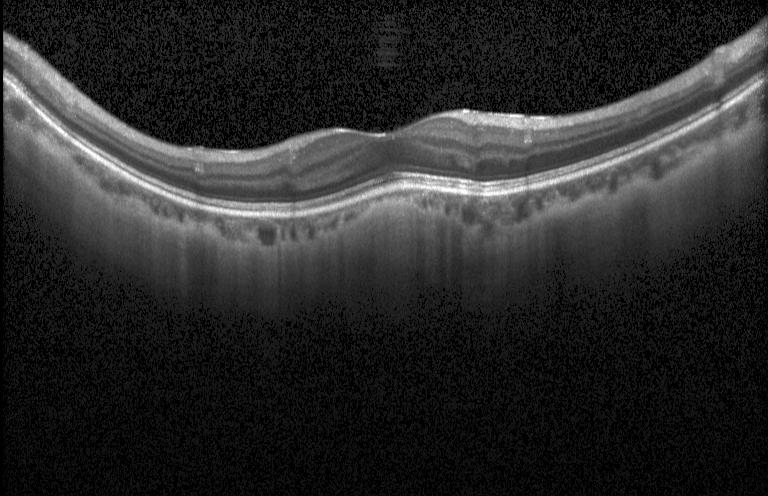
Optical coherence tomography B-scan; fovea-centered. Neither CNV, DME, nor drusen.